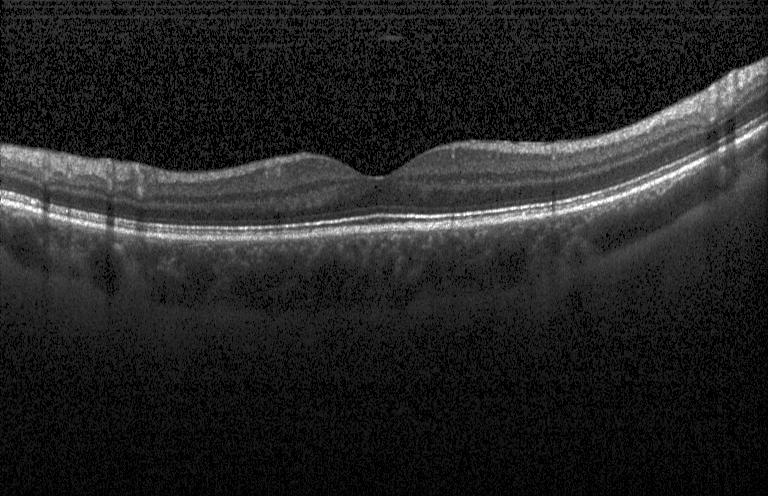
OCT line scan · macular scan.
Impression: no choroidal neovascularization, no diabetic macular edema, and no drusen.